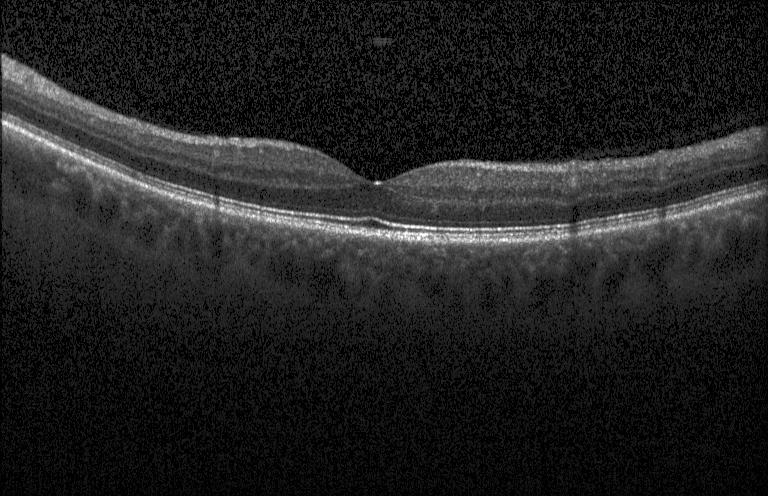 Centered on the fovea; spectral-domain optical coherence tomography; Heidelberg Spectralis OCT system; retinal OCT B-scan.
This B-scan demonstrates no choroidal neovascularization, no diabetic macular edema, and no drusen.